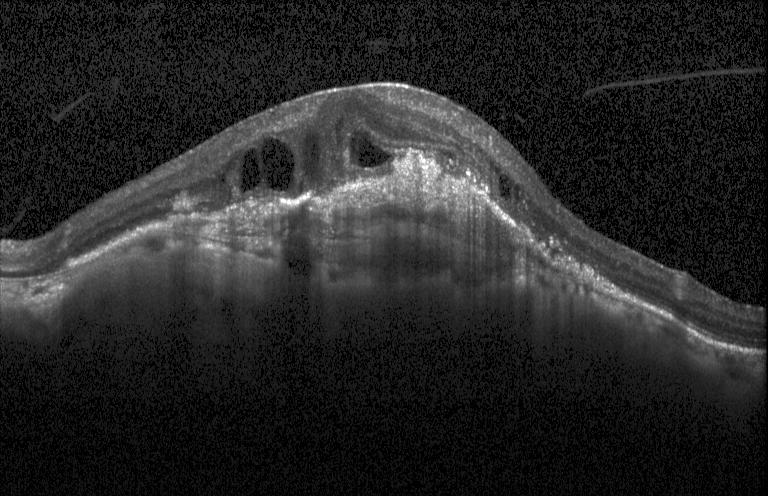 OCT B-scan · centered on the fovea — The scan shows a choroidal neovascular membrane.